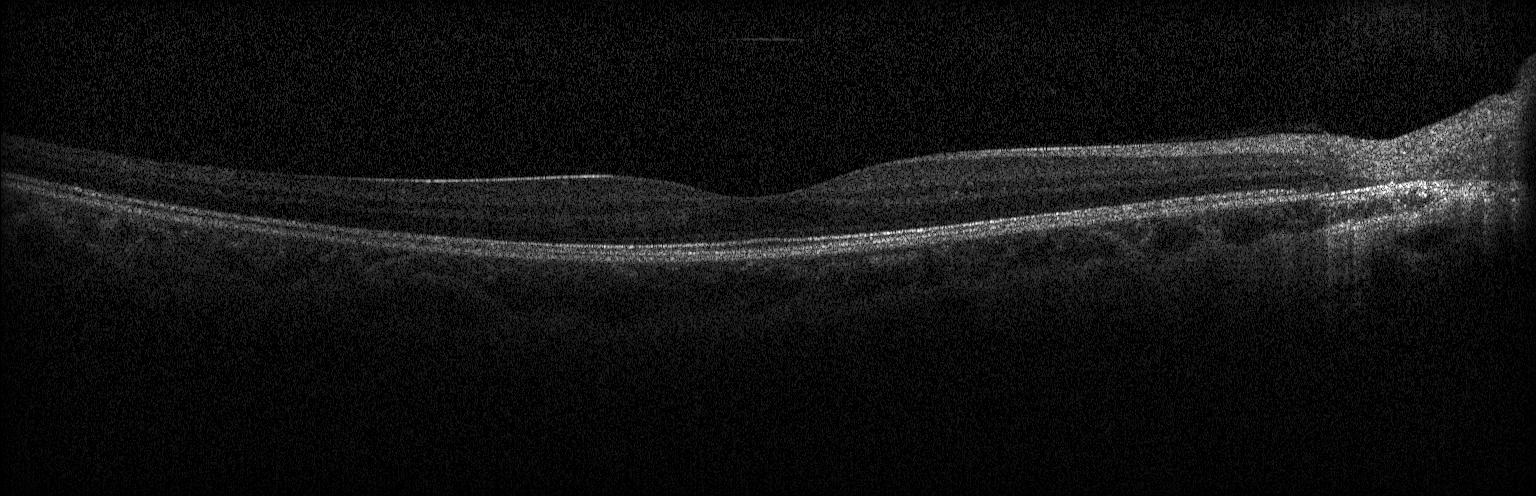 Instrument: Heidelberg Spectralis · retinal OCT cross-section · horizontal scan through the fovea · SD-OCT
No choroidal neovascularization, diabetic macular edema, or drusen.